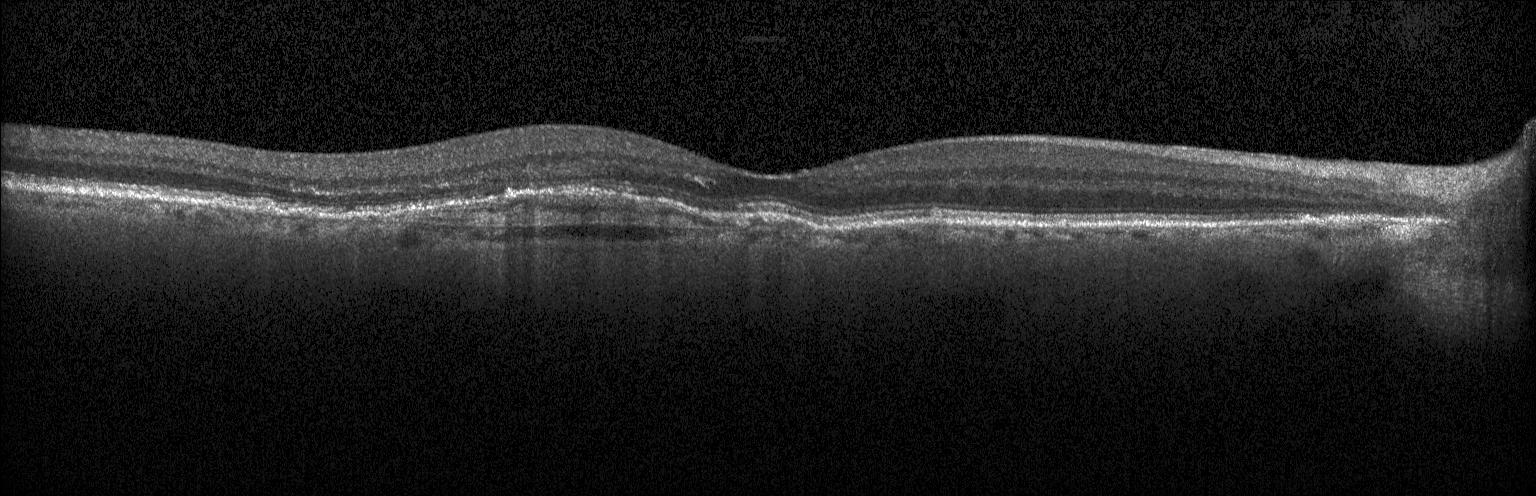 Instrument: Heidelberg Spectralis. OCT line scan — The scan shows choroidal neovascularization (CNV).